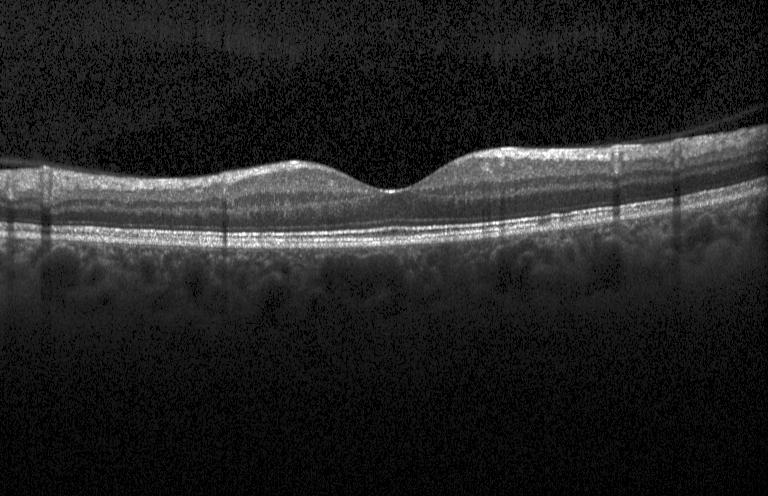 Retinal OCT cross-section.
Macular OCT: neither CNV, DME, nor drusen.